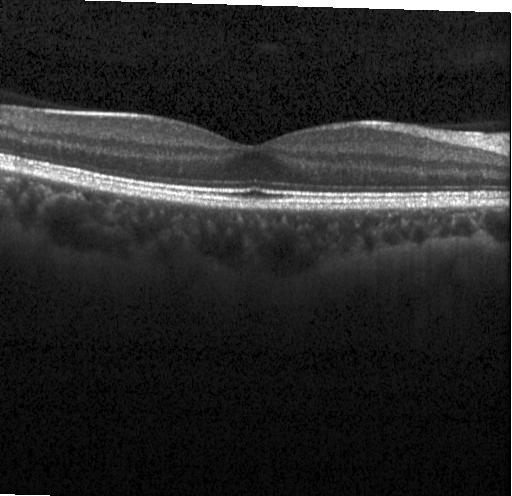

Centered on the fovea · optical coherence tomography B-scan.
Dx: no choroidal neovascularization, no diabetic macular edema, and no drusen.